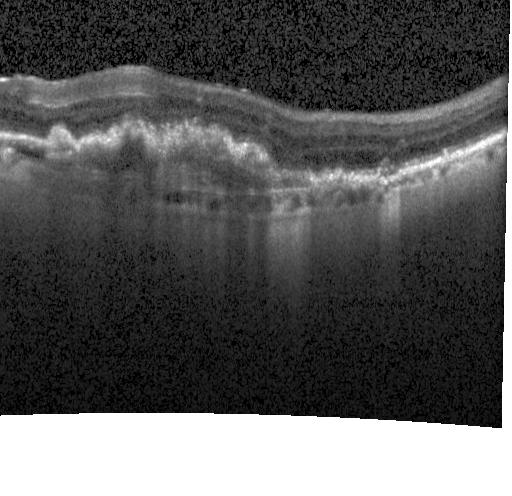

Dx: choroidal neovascularization (CNV).